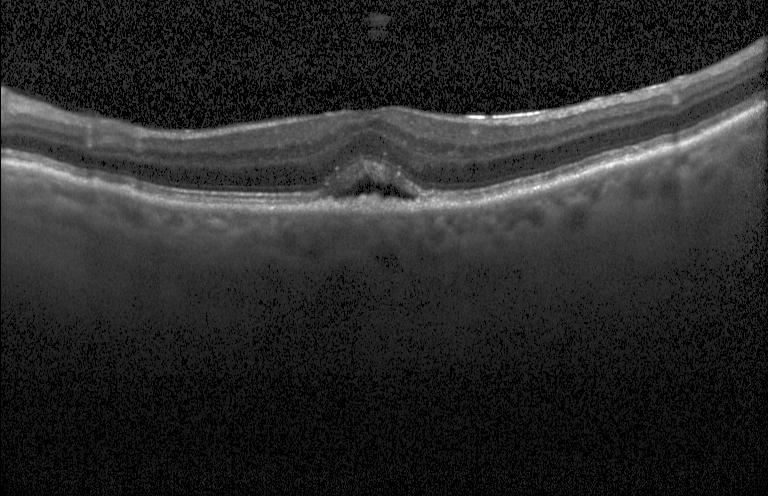

Diagnosis: choroidal neovascularization (CNV).